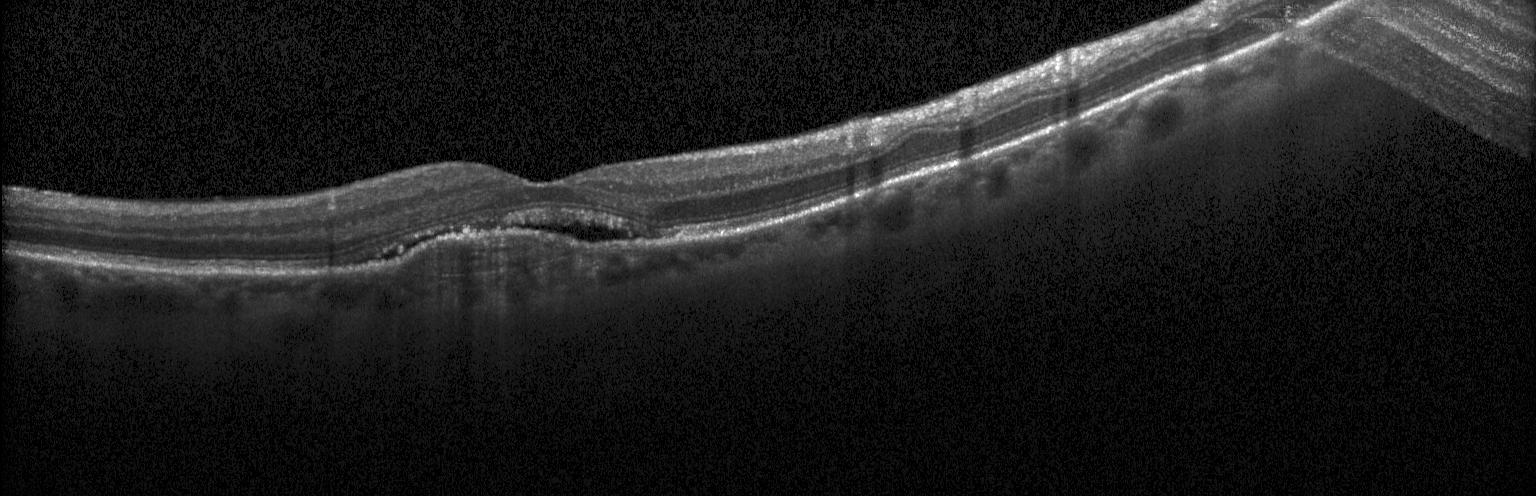

OCT B-scan; spectral-domain optical coherence tomography; centered on the fovea
Impression: choroidal neovascularization.